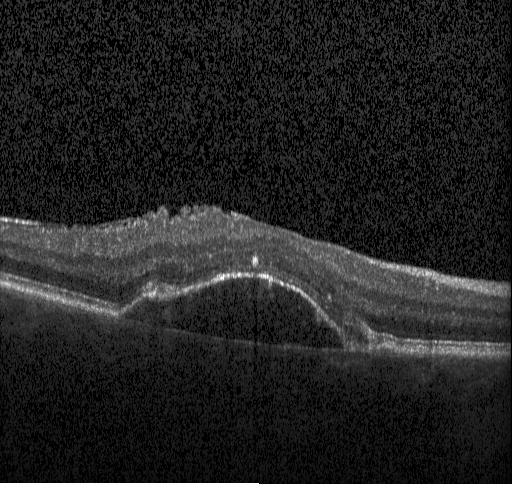 OCT line scan · spectral-domain optical coherence tomography · instrument: Heidelberg Spectralis · through the macula. Finding: a choroidal neovascular membrane.